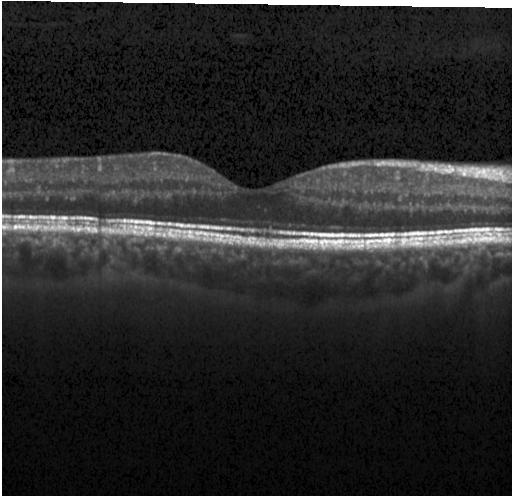
Heidelberg Spectralis. Horizontal scan through the fovea. Optical coherence tomography scan. Finding: neither choroidal neovascularization, diabetic macular edema, nor drusen.